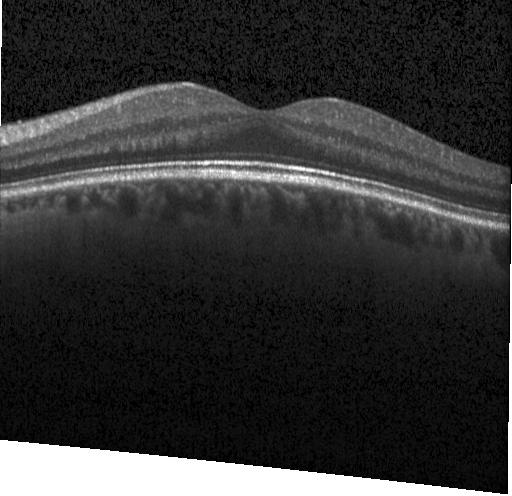

Finding: neither CNV, DME, nor drusen.